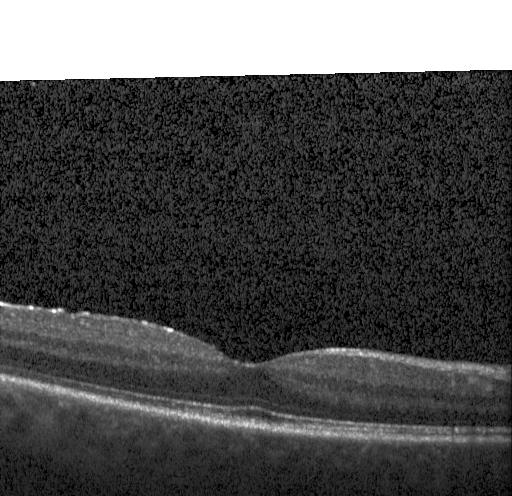 Macular OCT demonstrating no evidence of choroidal neovascularization, diabetic macular edema, or drusen.